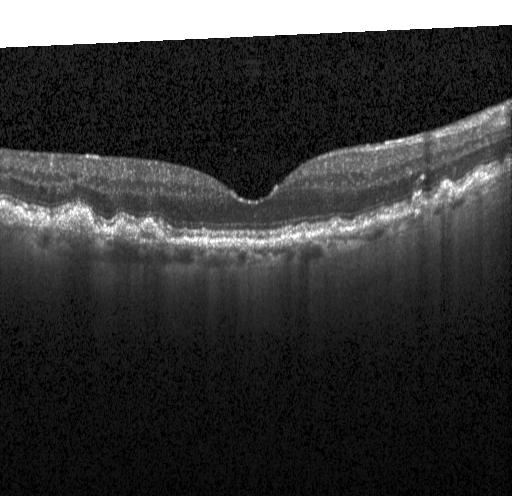 Macular scan. SD-OCT. Retinal OCT cross-section
Impression: sub-RPE drusenoid deposits.